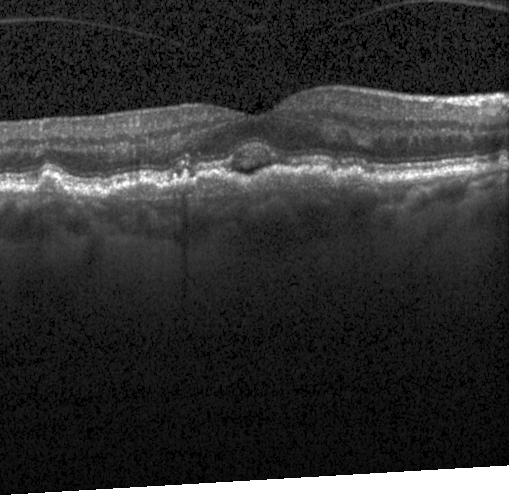
Optical coherence tomography scan · horizontal scan through the fovea · Heidelberg Spectralis · SD-OCT — Diagnosis: a choroidal neovascular membrane.